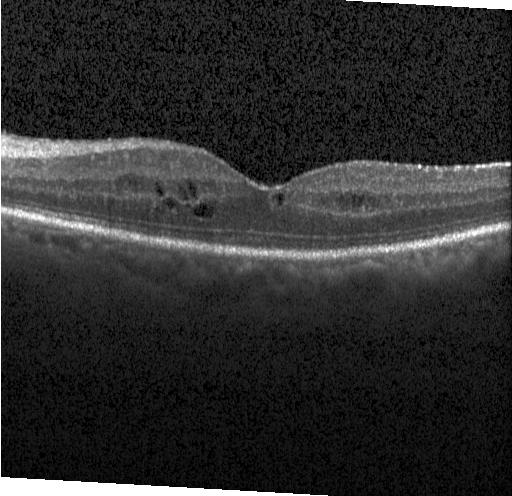

OCT finding: diabetic macular edema.